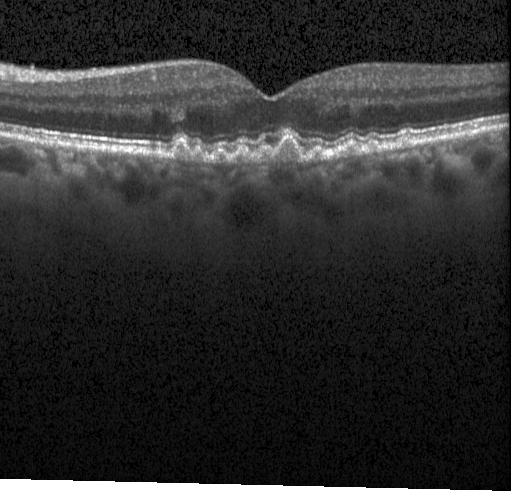
Heidelberg Spectralis, spectral-domain optical coherence tomography, through the macula, retinal OCT B-scan — Finding: multiple drusen.